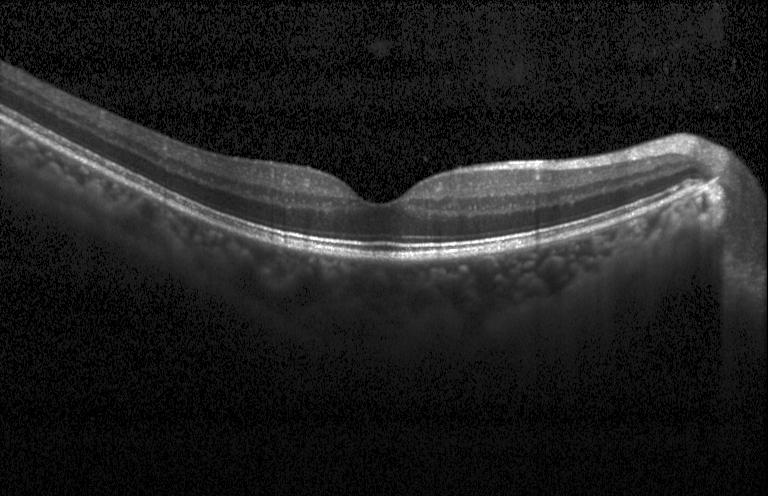 The scan shows neither CNV, DME, nor drusen.